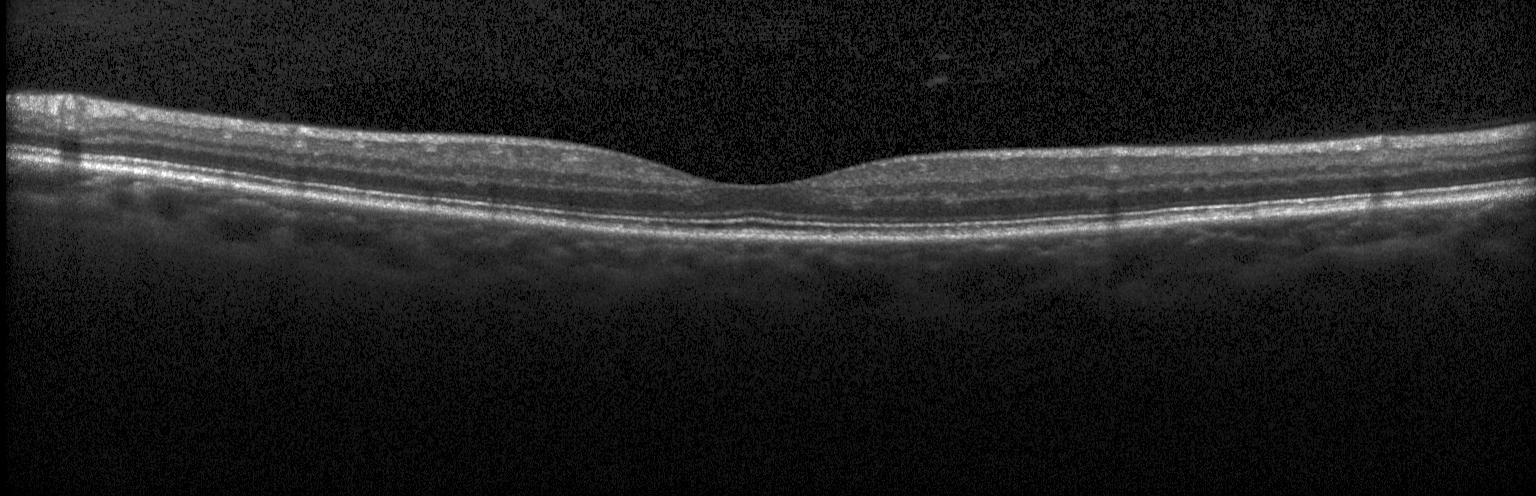

Impression: no choroidal neovascularization, diabetic macular edema, or drusen.